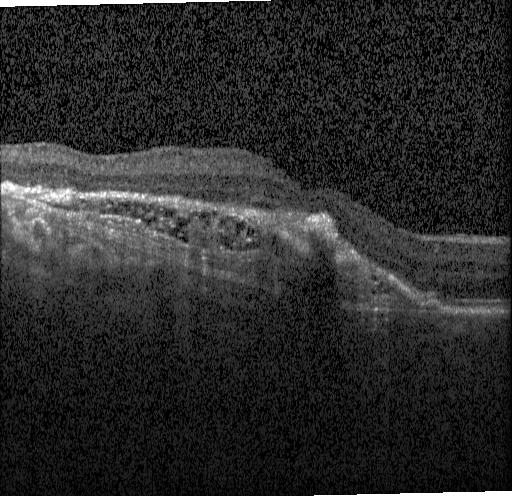
Impression: choroidal neovascularization (CNV).